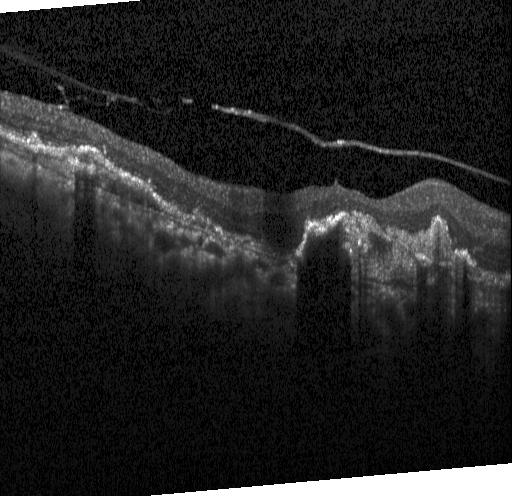
Centered on the fovea; spectral-domain OCT; optical coherence tomography scan; Heidelberg Spectralis — Assessment: CNV.